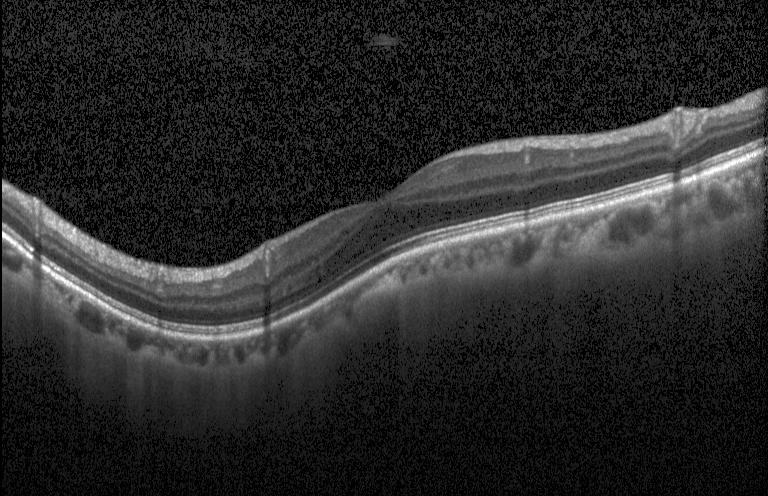
OCT B-scan — Diagnosis: no CNV, no DME, and no drusen.